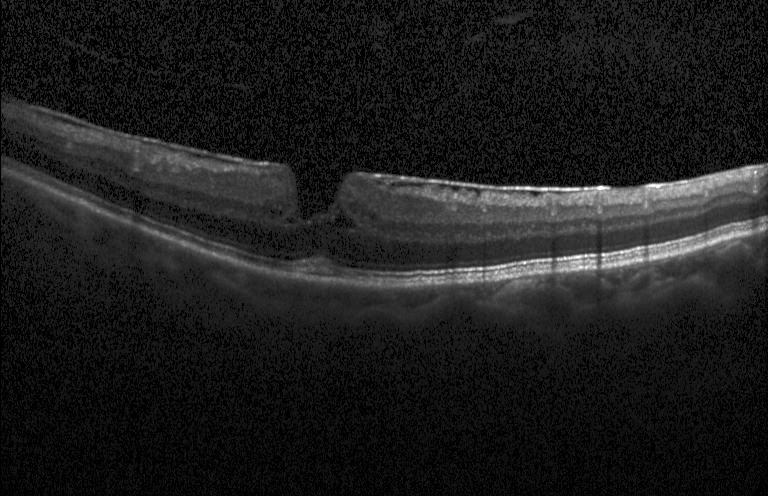

OCT B-scan — Diagnosis: diabetic macular edema (DME).